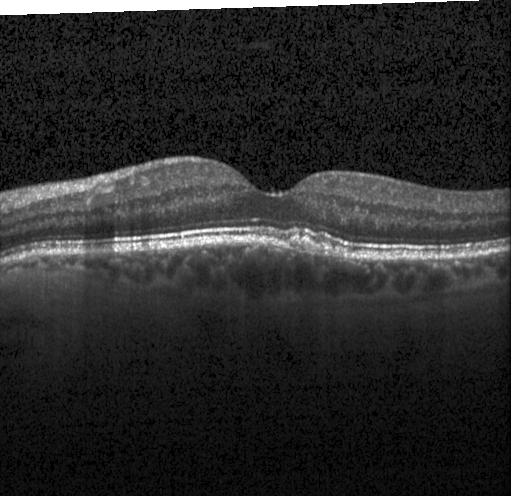

Diagnosis: sub-RPE drusenoid deposits.